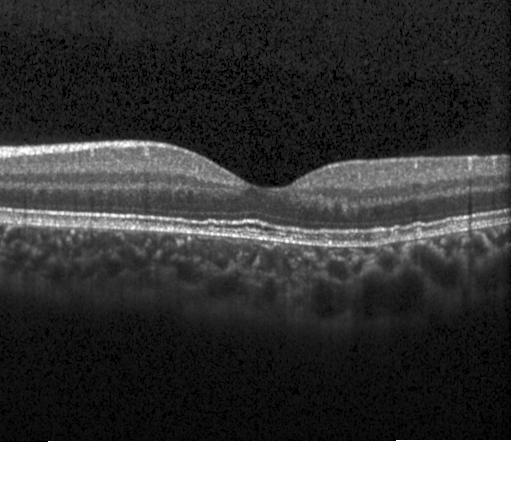 Retinal OCT B-scan. Acquired on a Heidelberg Spectralis. SD-OCT.
Assessment: no choroidal neovascularization, no diabetic macular edema, and no drusen.